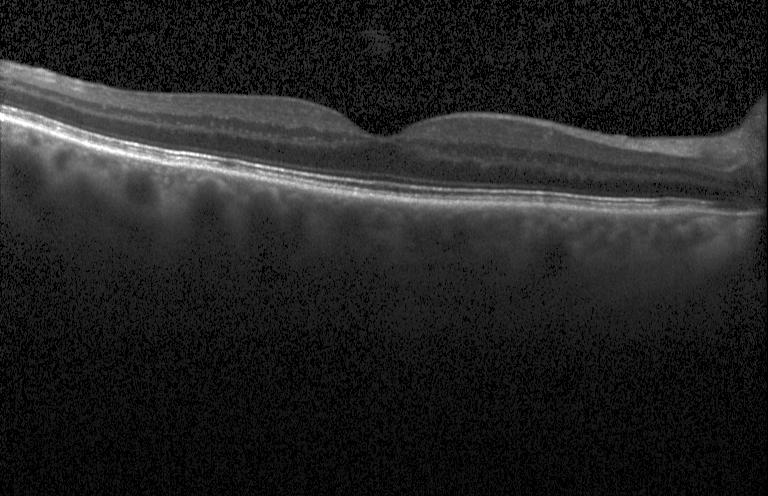

Optical coherence tomography scan, SD-OCT.
Macular OCT: neither choroidal neovascularization, diabetic macular edema, nor drusen.